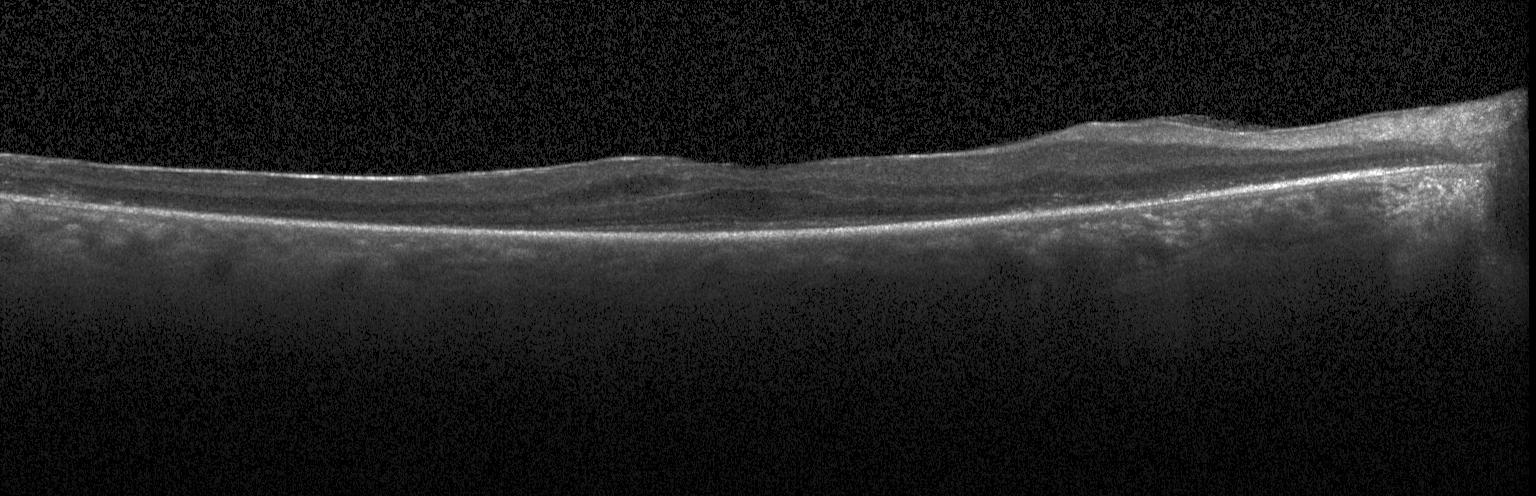 Macular scan · Heidelberg Spectralis OCT system · optical coherence tomography scan · spectral-domain optical coherence tomography. Dx: diabetic macular edema (DME).